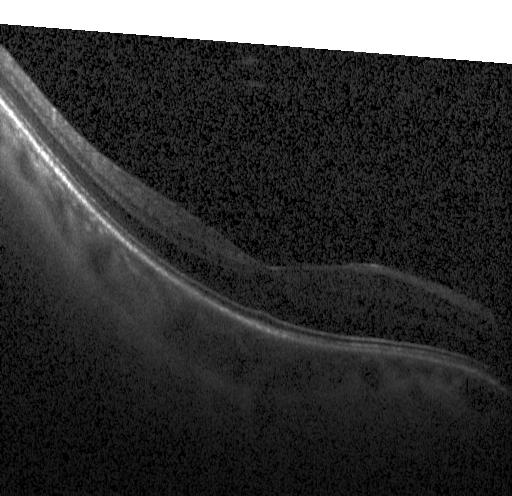 Acquired on a Heidelberg Spectralis. OCT line scan. Spectral-domain optical coherence tomography. Diagnosis: neither choroidal neovascularization, diabetic macular edema, nor drusen.